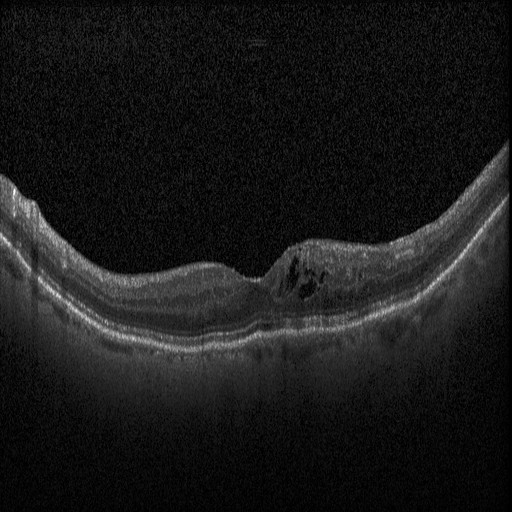

Spectral-domain optical coherence tomography; acquired on a Heidelberg Spectralis; macular scan; optical coherence tomography scan — Finding: diabetic macular edema (DME).